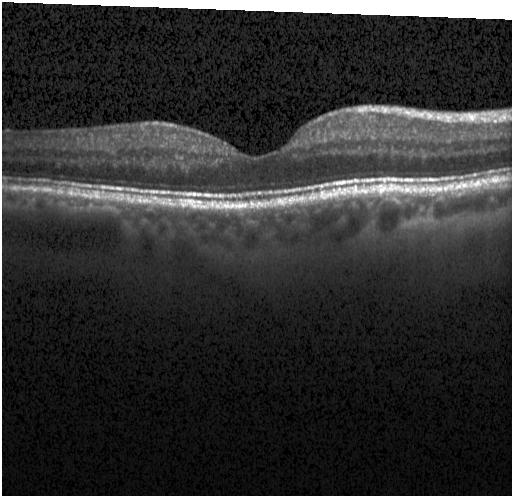
Retinal OCT cross-section. Diagnosis: no CNV, no DME, and no drusen.